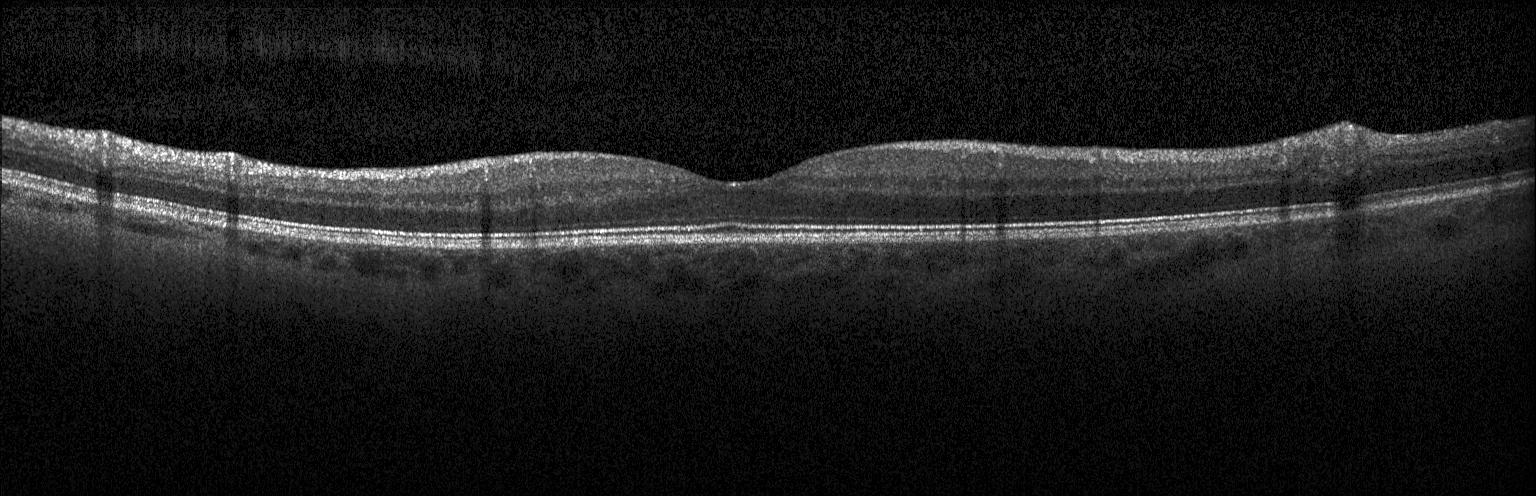 Retinal OCT cross-section. Instrument: Heidelberg Spectralis — Impression: no CNV, DME, or drusen.